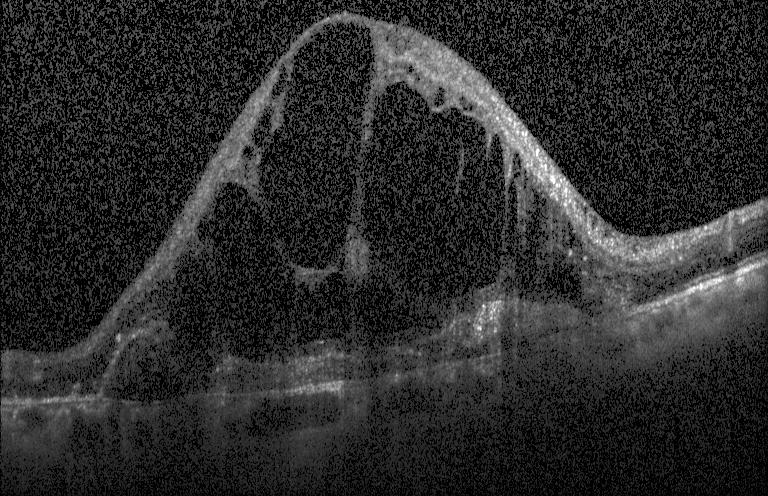 OCT finding: a choroidal neovascular membrane.